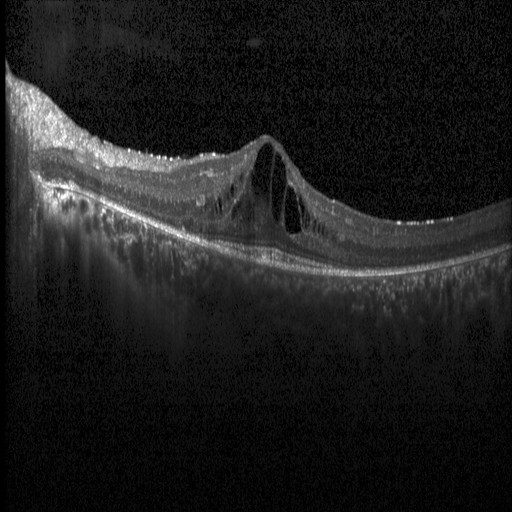 OCT B-scan — Finding: diabetic macular edema (DME).